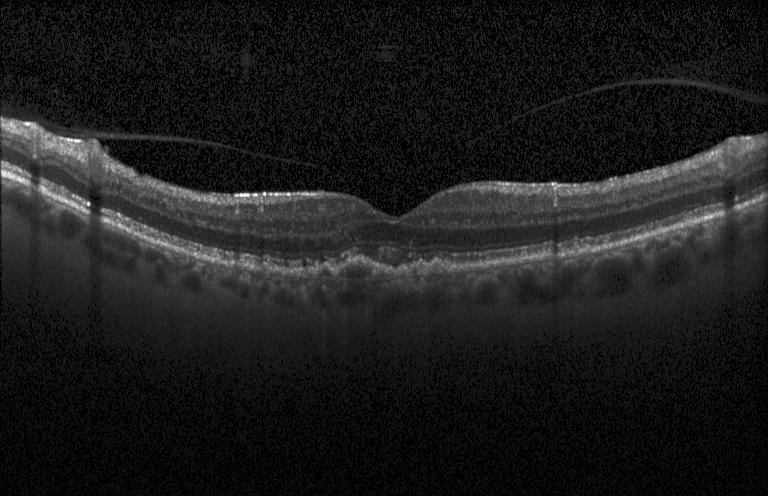 Spectral-domain optical coherence tomography. Optical coherence tomography B-scan. Instrument: Heidelberg Spectralis. Centered on the fovea.
The scan shows a choroidal neovascular membrane.